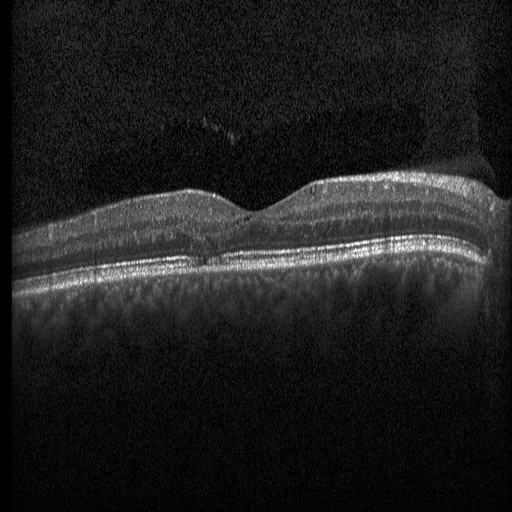 Optical coherence tomography B-scan, horizontal scan through the fovea, SD-OCT
Dx: diabetic macular edema (DME).